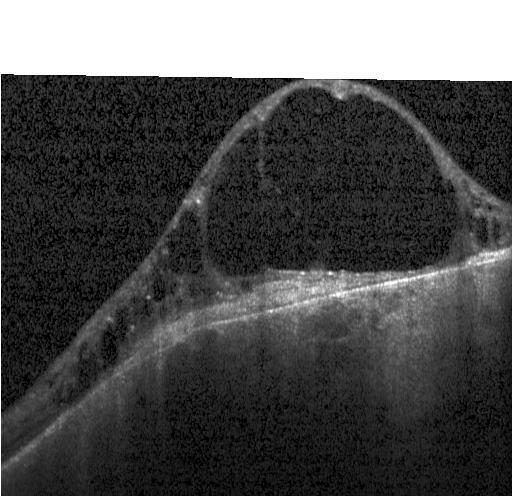 This B-scan demonstrates a choroidal neovascular membrane.